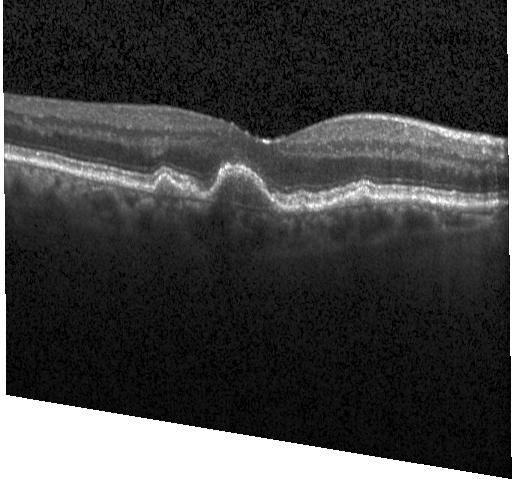 Macular OCT demonstrating sub-RPE drusenoid deposits.